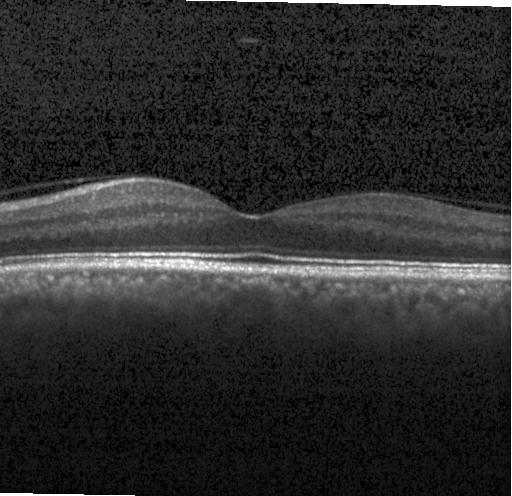 Retinal OCT cross-section showing neither choroidal neovascularization, diabetic macular edema, nor drusen.